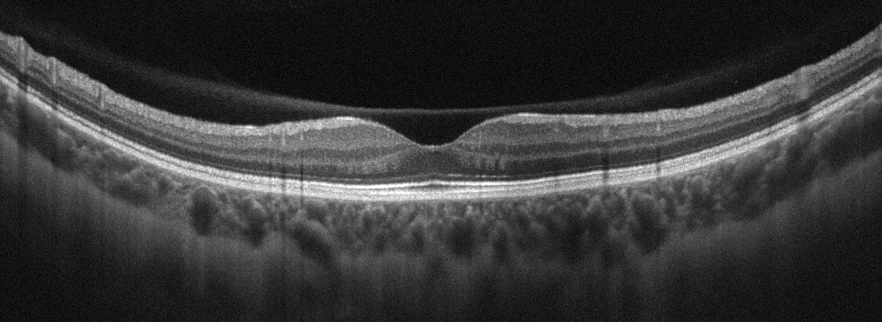
Optical coherence tomography B-scan. Diagnosis: absence of AMD, DME, ERM, RAO, RVO, and vitreomacular interface disease.